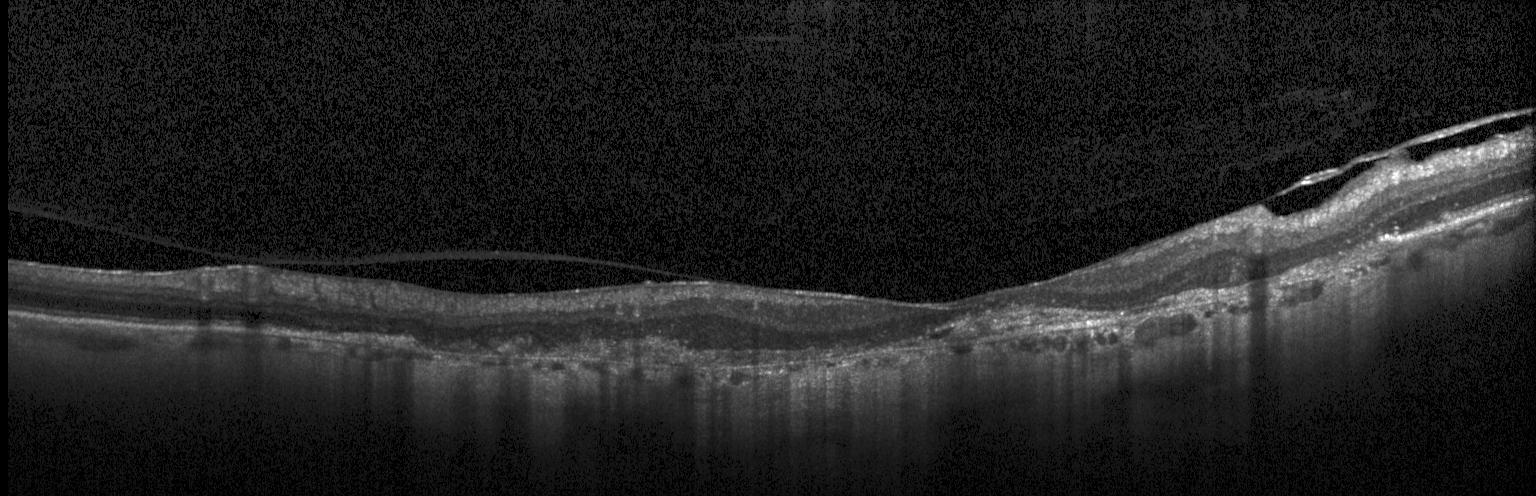
Macular scan. OCT line scan. Heidelberg Spectralis OCT system
Impression: a choroidal neovascular membrane.